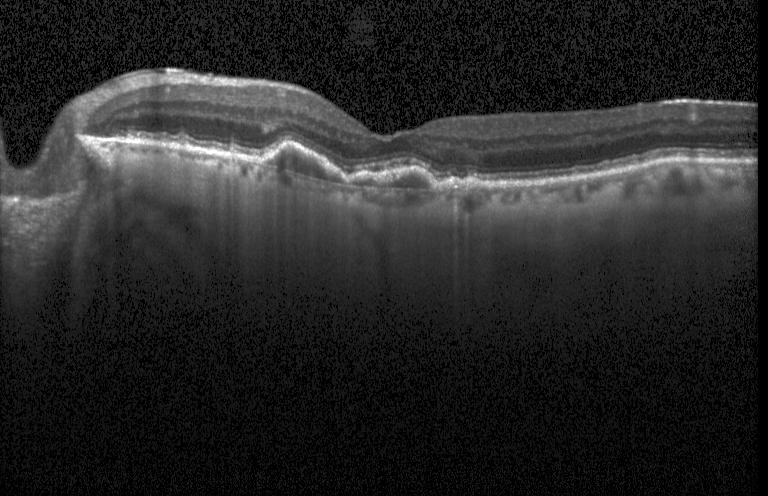 The scan shows a choroidal neovascular membrane.